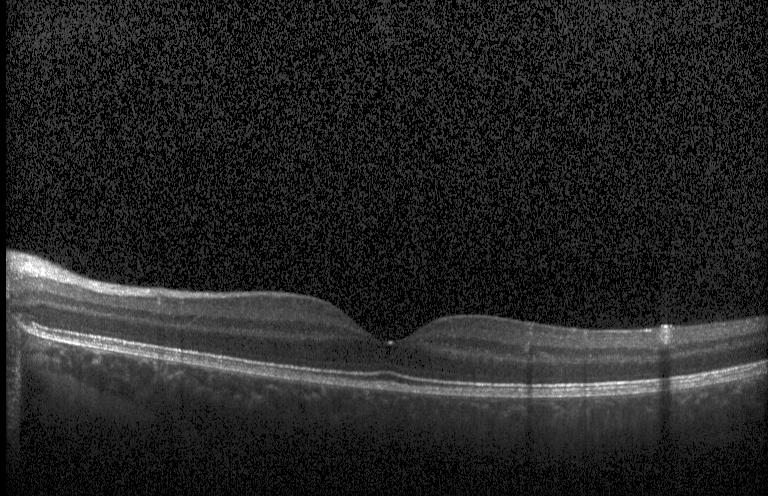 OCT line scan, acquired on a Heidelberg Spectralis — This B-scan demonstrates no choroidal neovascularization, no diabetic macular edema, and no drusen.